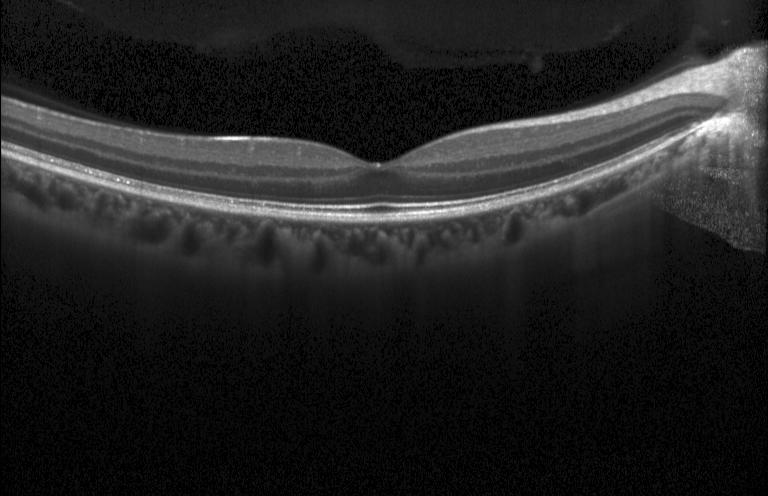

OCT line scan — Assessment: no CNV, no DME, and no drusen.